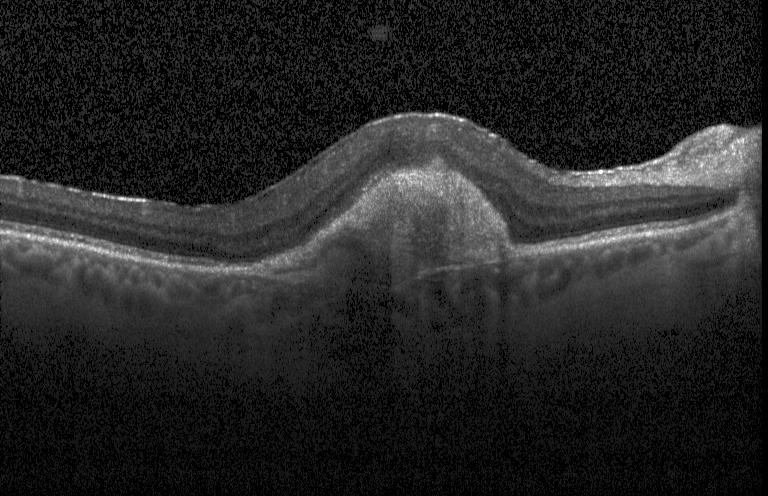 Retinal OCT B-scan.
Diagnosis: choroidal neovascularization.